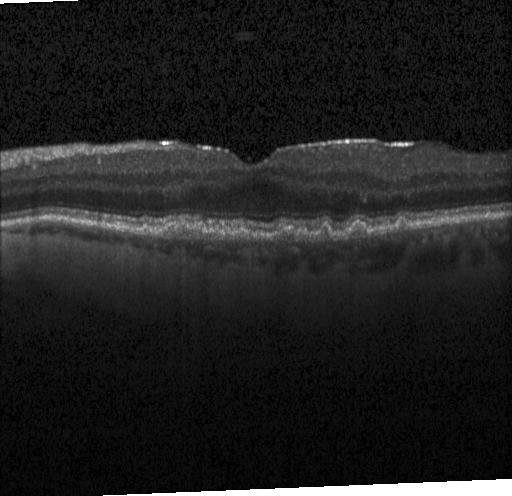

Drusen.